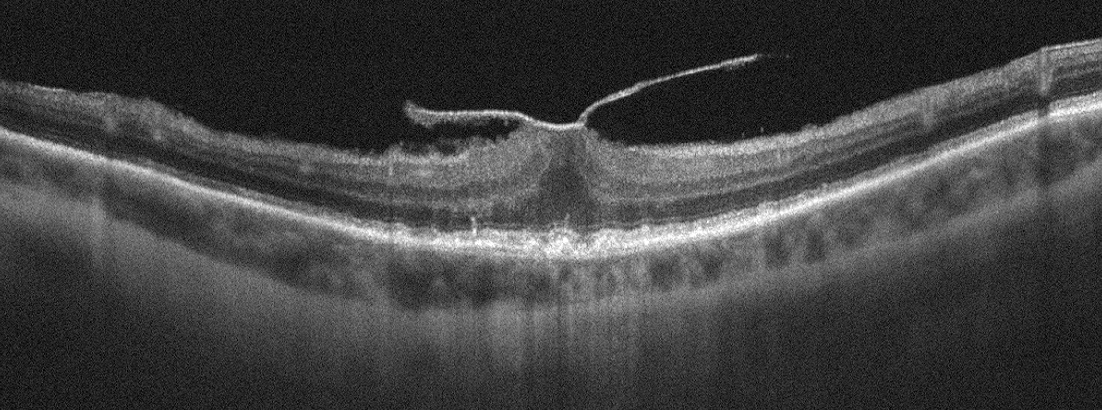 OCT scan showing epiretinal membrane (ERM).